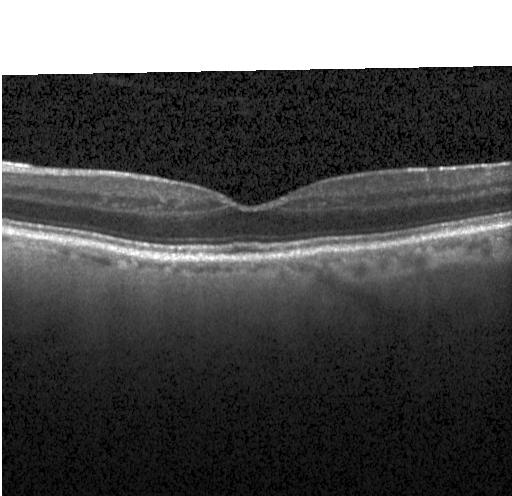

SD-OCT · Heidelberg Spectralis OCT system · retinal OCT B-scan.
This B-scan demonstrates no CNV, DME, or drusen.